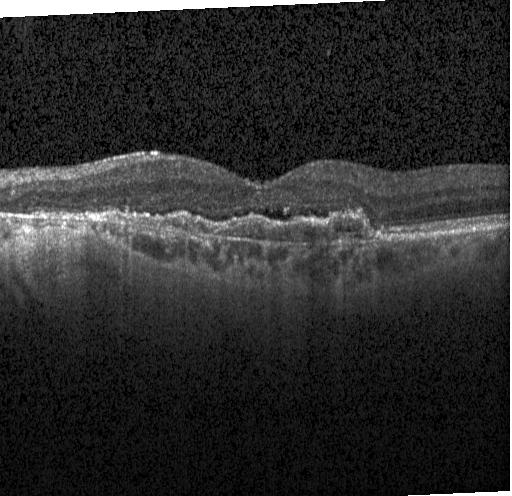 Heidelberg Spectralis OCT system, optical coherence tomography B-scan.
OCT finding: choroidal neovascularization (CNV).